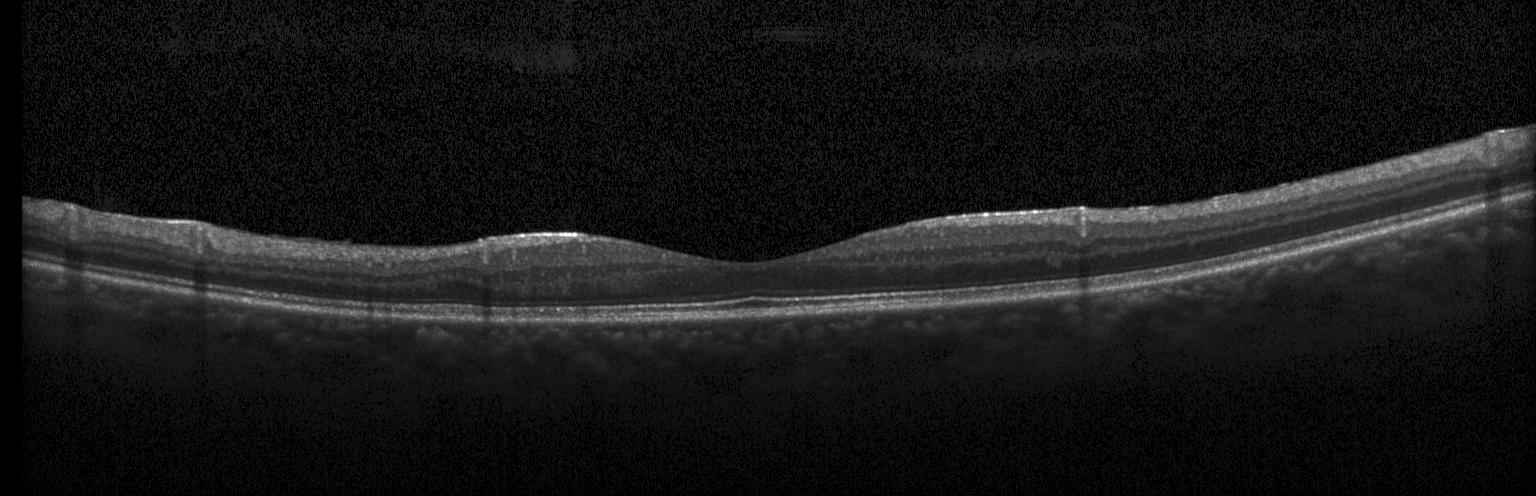

Retinal OCT cross-section; fovea-centered — Neither CNV, DME, nor drusen.